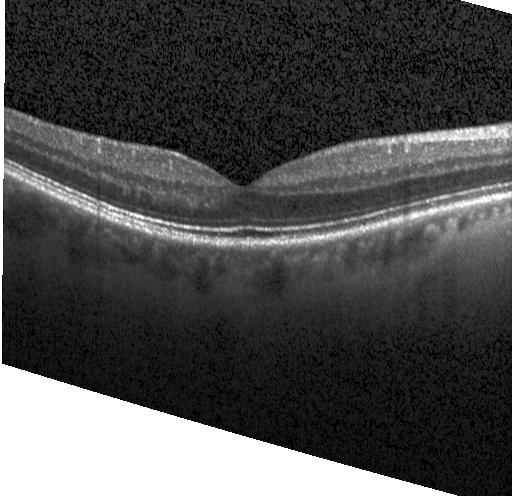

Heidelberg Spectralis OCT system · spectral-domain OCT · horizontal scan through the fovea · retinal OCT cross-section. The scan shows no evidence of choroidal neovascularization, diabetic macular edema, or drusen.